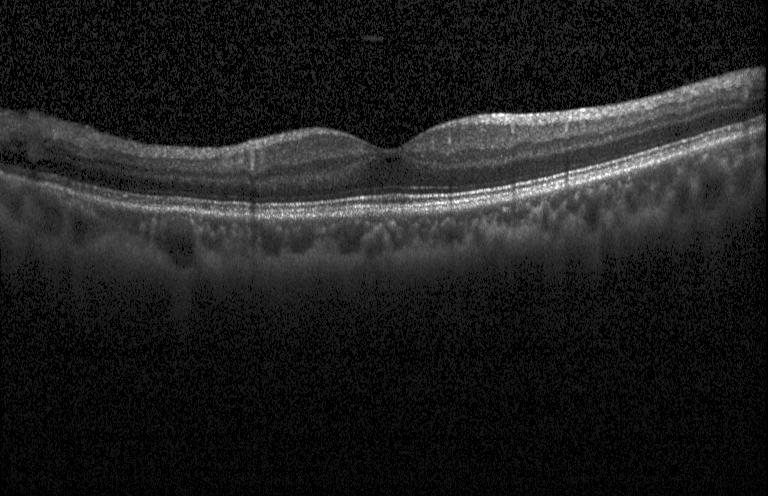 Retinal OCT B-scan; through the macula; Heidelberg Spectralis; spectral-domain optical coherence tomography.
This B-scan demonstrates no evidence of choroidal neovascularization, diabetic macular edema, or drusen.